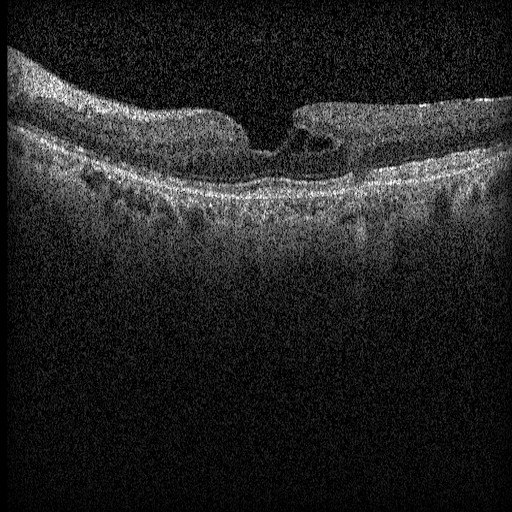
SD-OCT, acquired on a Heidelberg Spectralis, retinal OCT cross-section
OCT finding: diabetic macular edema (DME).